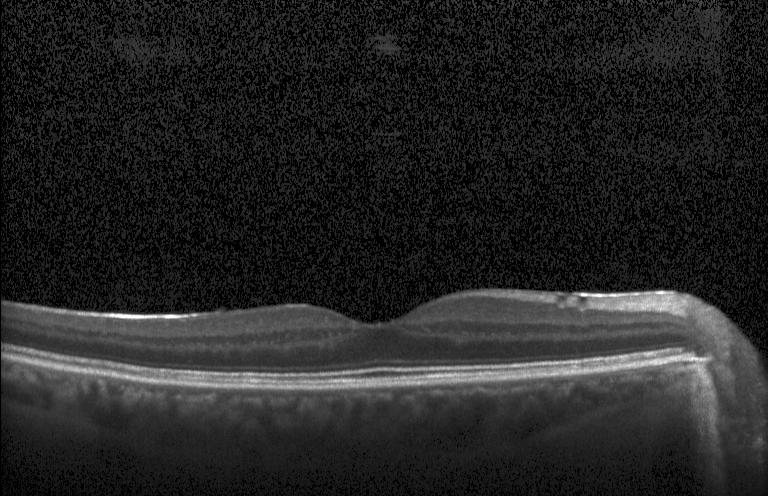
Diagnosis: no choroidal neovascularization, diabetic macular edema, or drusen.